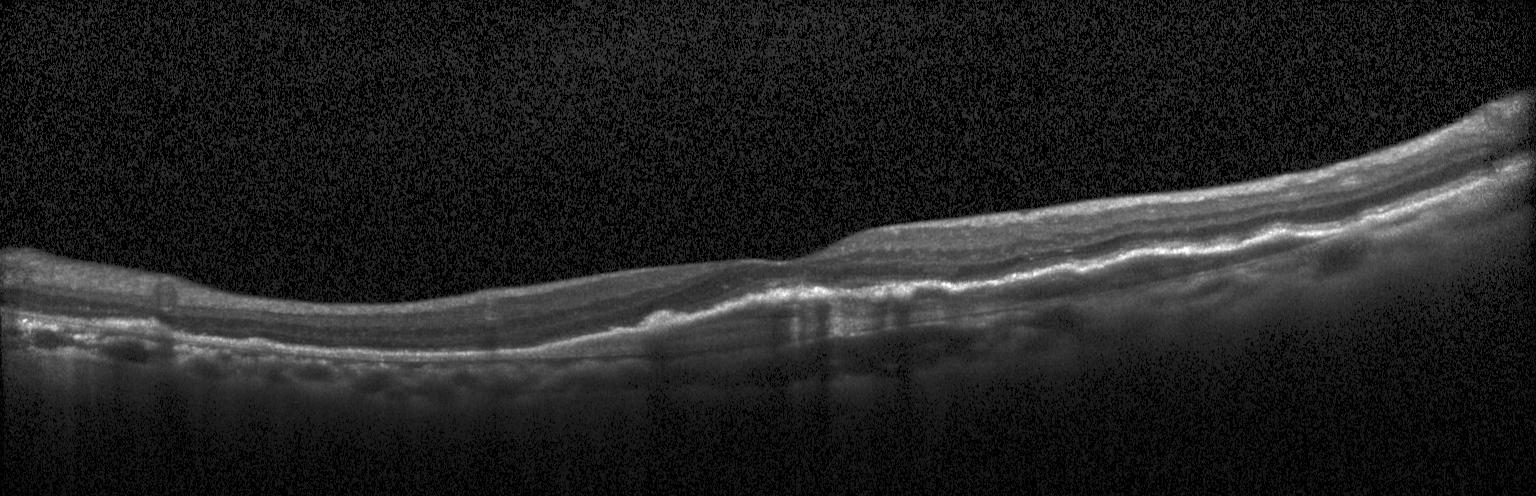

Retinal OCT cross-section
OCT finding: choroidal neovascularization (CNV).